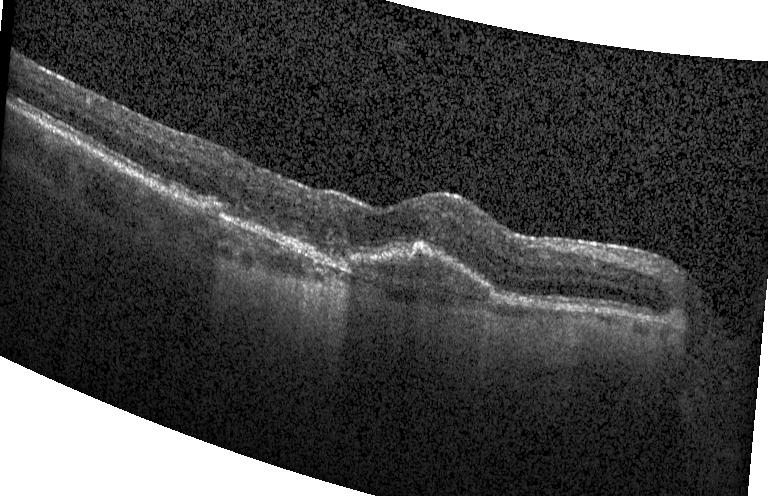 Retinal OCT cross-section — Finding: a choroidal neovascular membrane.